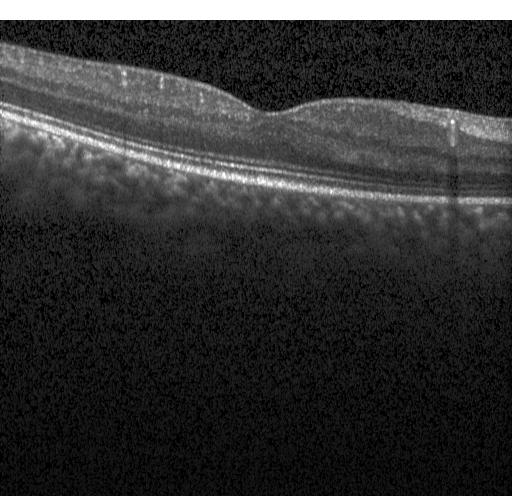 Fovea-centered. Optical coherence tomography B-scan. Spectral-domain optical coherence tomography.
This B-scan demonstrates no CNV, DME, or drusen.